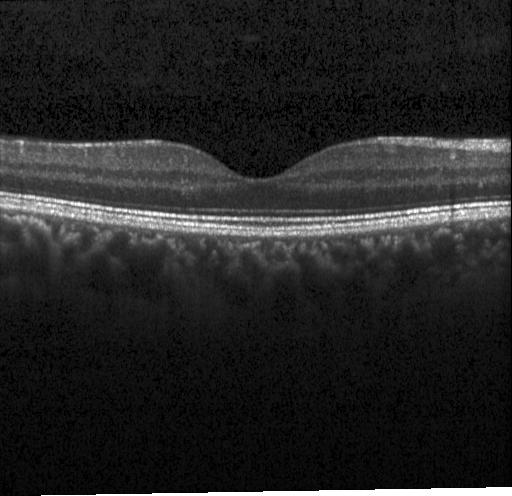 Optical coherence tomography B-scan. Spectral-domain optical coherence tomography. Fovea-centered. Instrument: Heidelberg Spectralis
Assessment: neither choroidal neovascularization, diabetic macular edema, nor drusen.